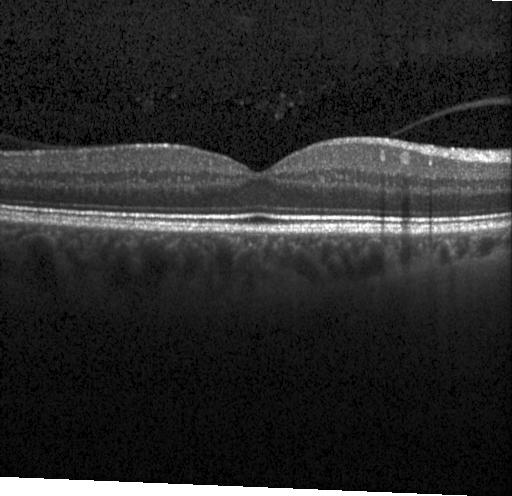

The scan shows no CNV, no DME, and no drusen.